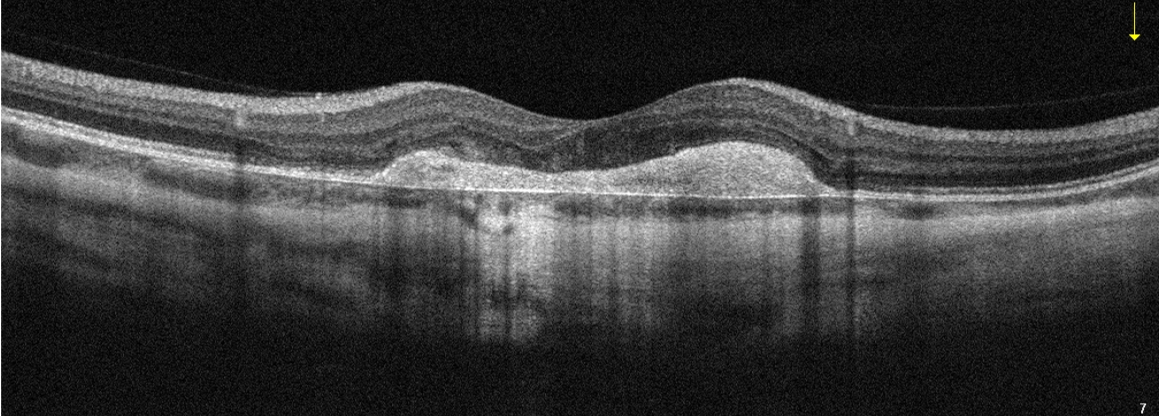

Impression: AMD.